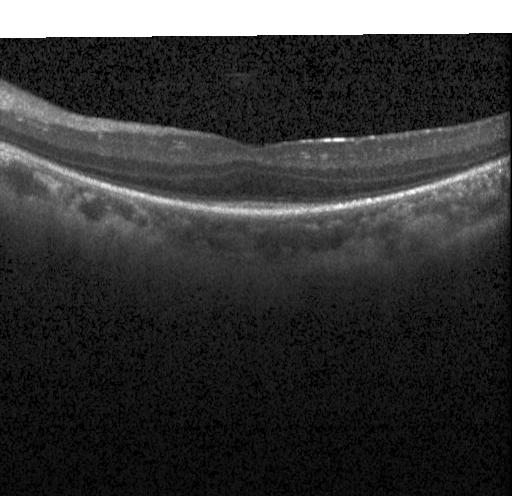

Retinal OCT B-scan · fovea-centered · Heidelberg Spectralis. Impression: no choroidal neovascularization, diabetic macular edema, or drusen.